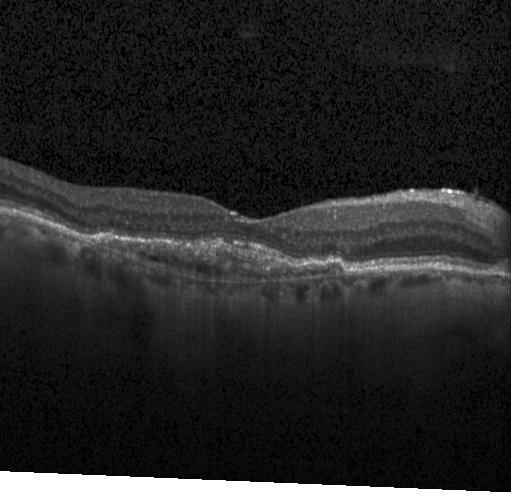

Through the macula · OCT line scan · spectral-domain optical coherence tomography.
The scan shows CNV.